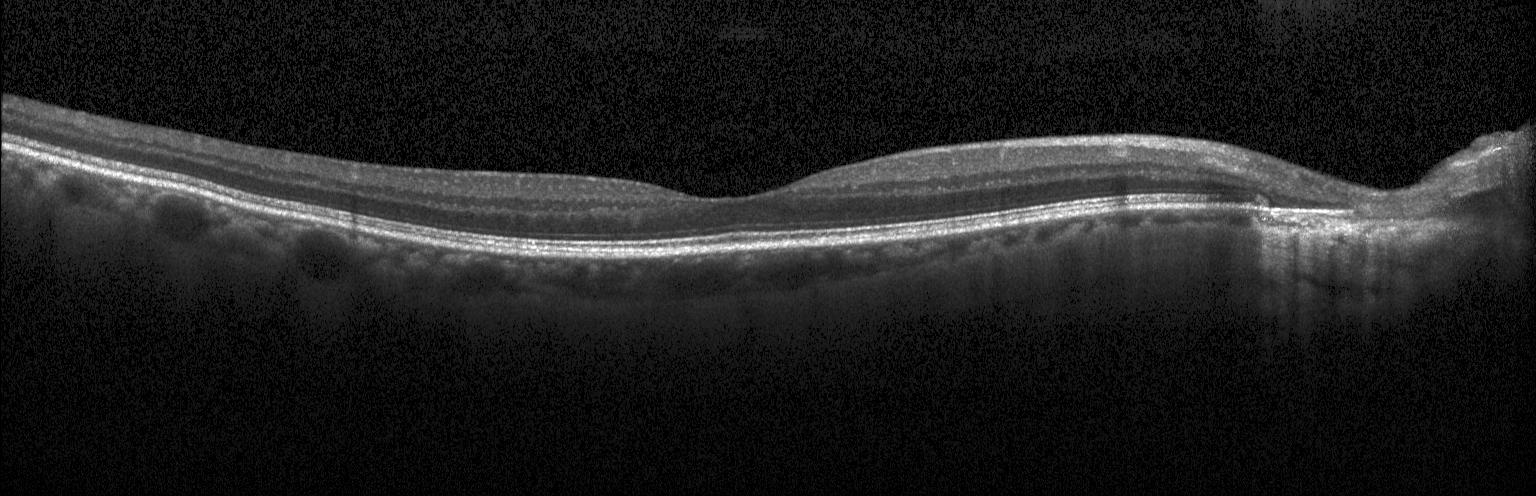
Optical coherence tomography B-scan; spectral-domain optical coherence tomography; Heidelberg Spectralis; fovea-centered.
Assessment: no CNV, no DME, and no drusen.